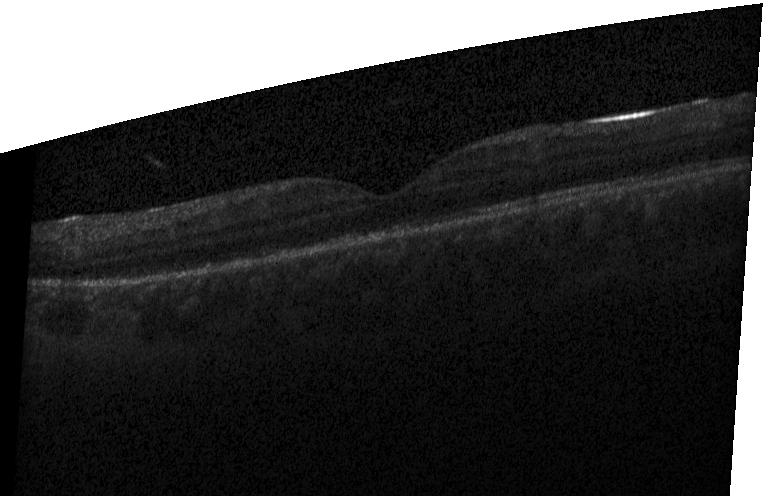

Optical coherence tomography scan
Finding: no CNV, no DME, and no drusen.